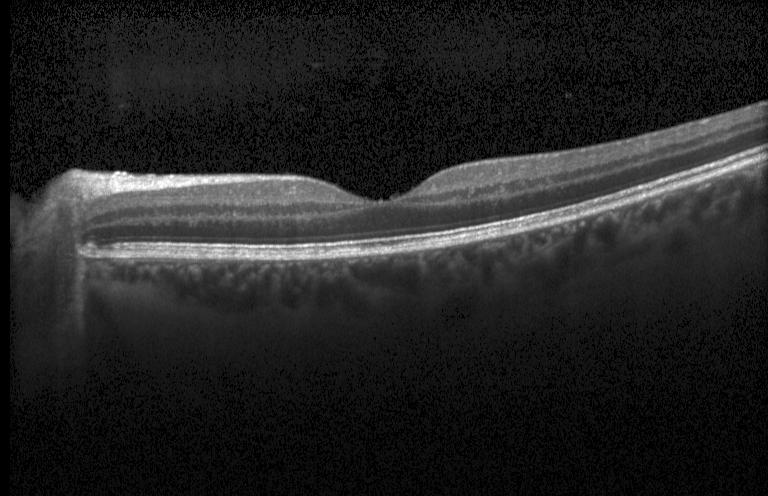

Assessment: no choroidal neovascularization, diabetic macular edema, or drusen.